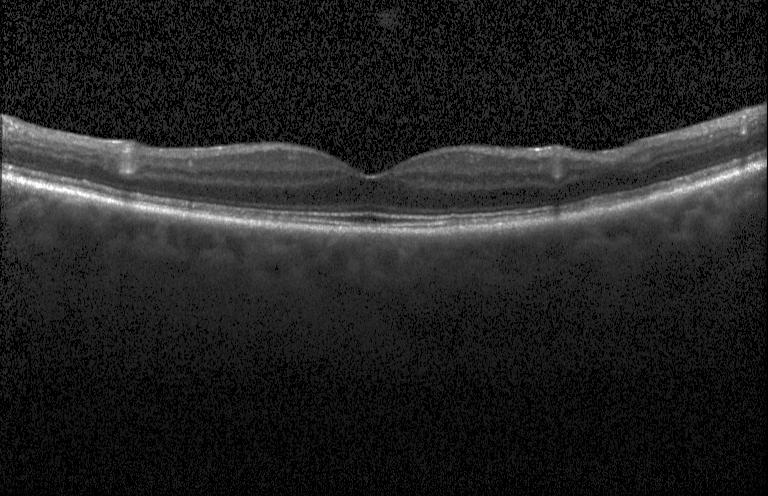

Heidelberg Spectralis OCT system. Retinal OCT cross-section.
Dx: no CNV, no DME, and no drusen.